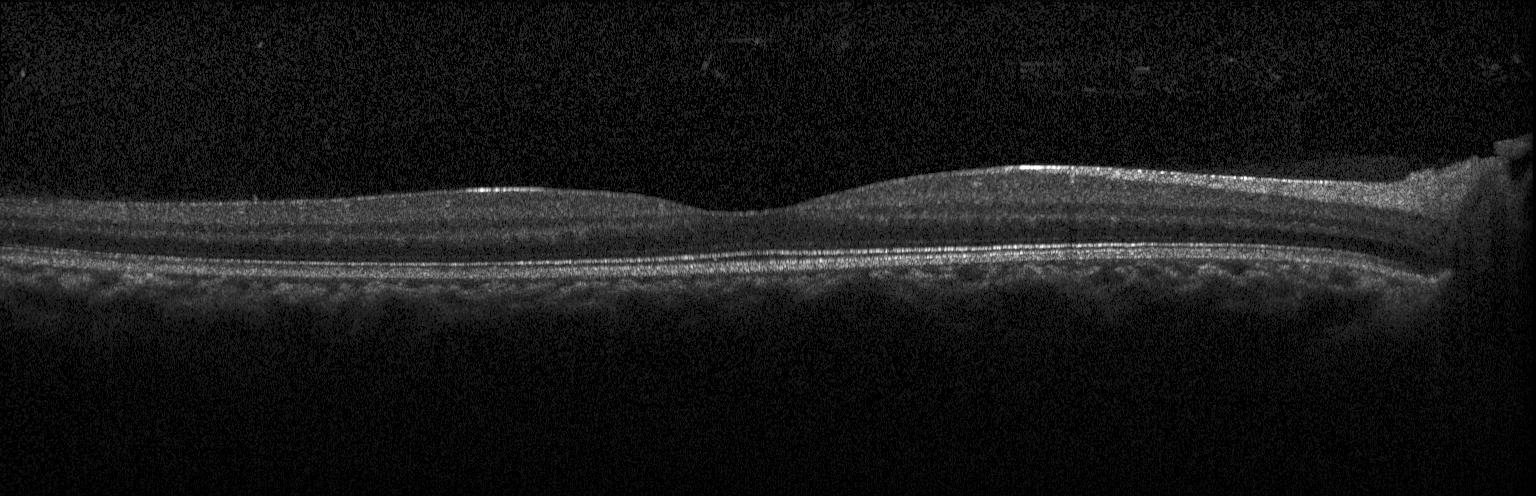 OCT finding: no evidence of choroidal neovascularization, diabetic macular edema, or drusen.